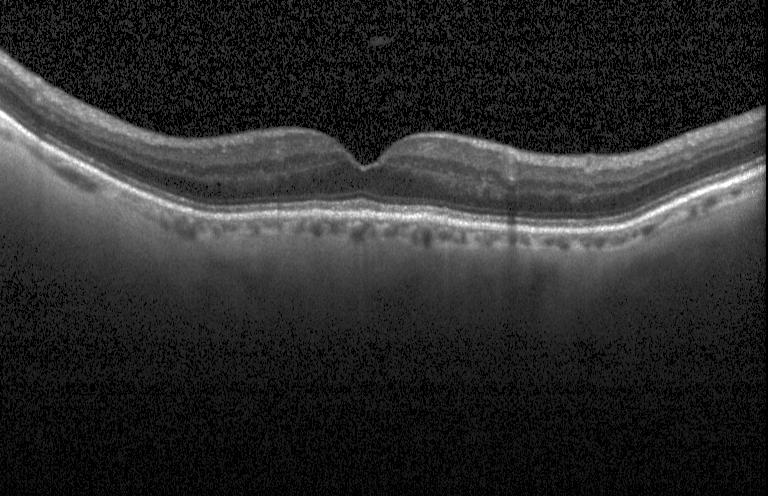
Dx: no evidence of choroidal neovascularization, diabetic macular edema, or drusen.